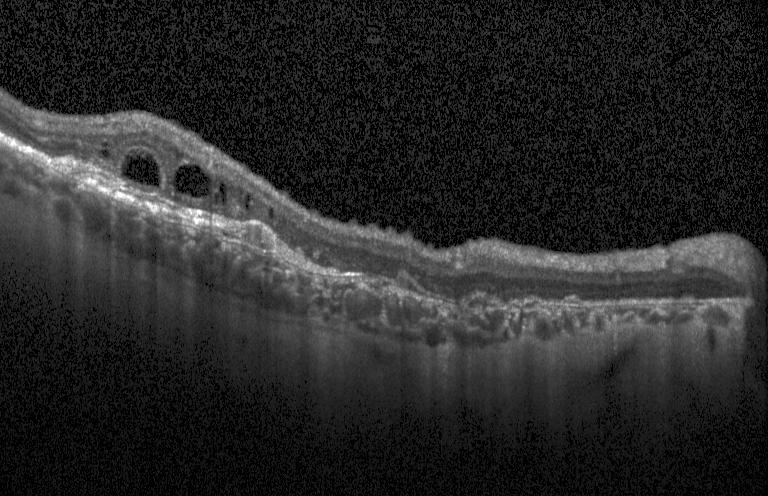 The scan shows a choroidal neovascular membrane.